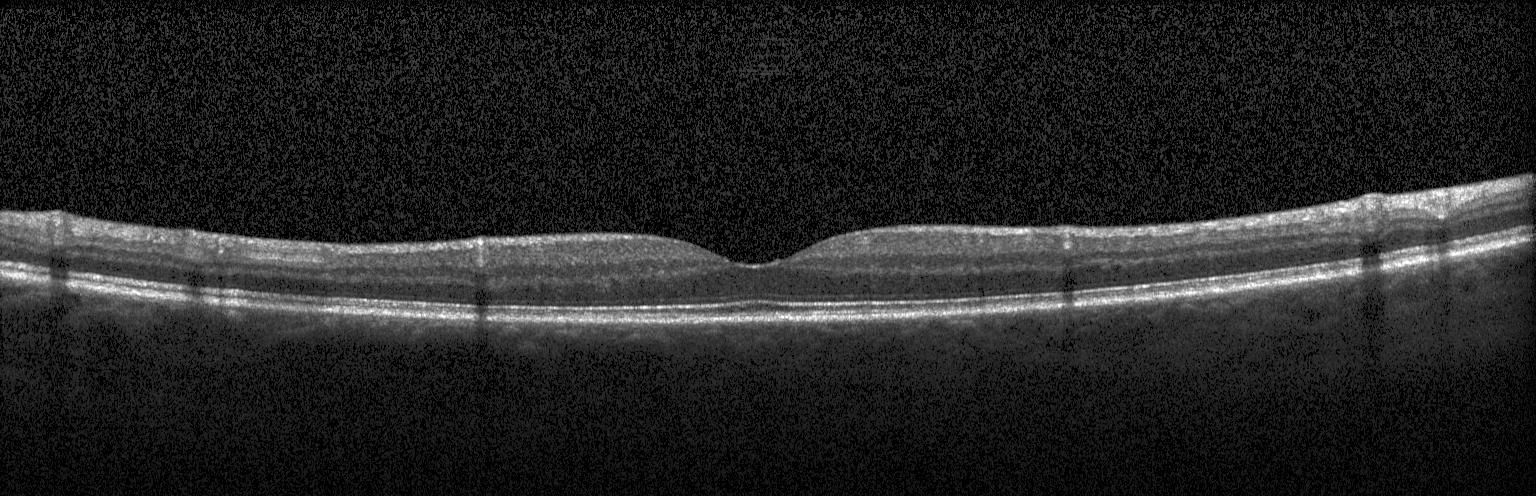

Spectral-domain optical coherence tomography. Fovea-centered. Acquired on a Heidelberg Spectralis. Retinal OCT cross-section
Assessment: no evidence of CNV, DME, or drusen.